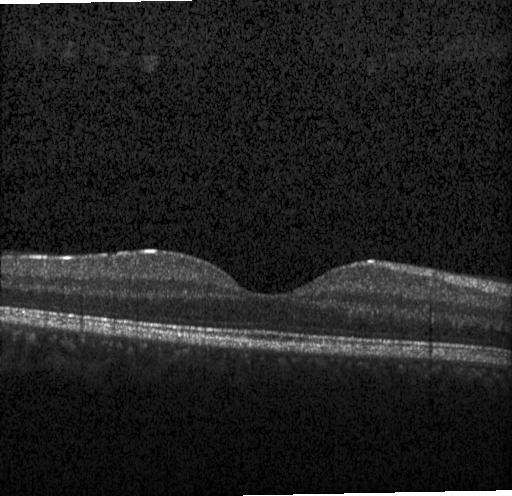 OCT B-scan. Centered on the fovea.
Diagnosis: no evidence of choroidal neovascularization, diabetic macular edema, or drusen.